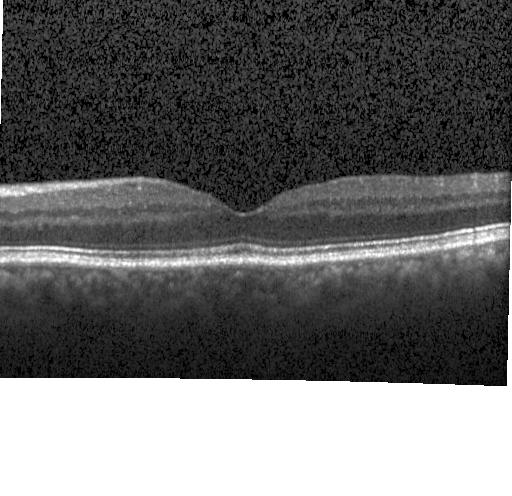
SD-OCT, optical coherence tomography B-scan.
Diagnosis: neither CNV, DME, nor drusen.